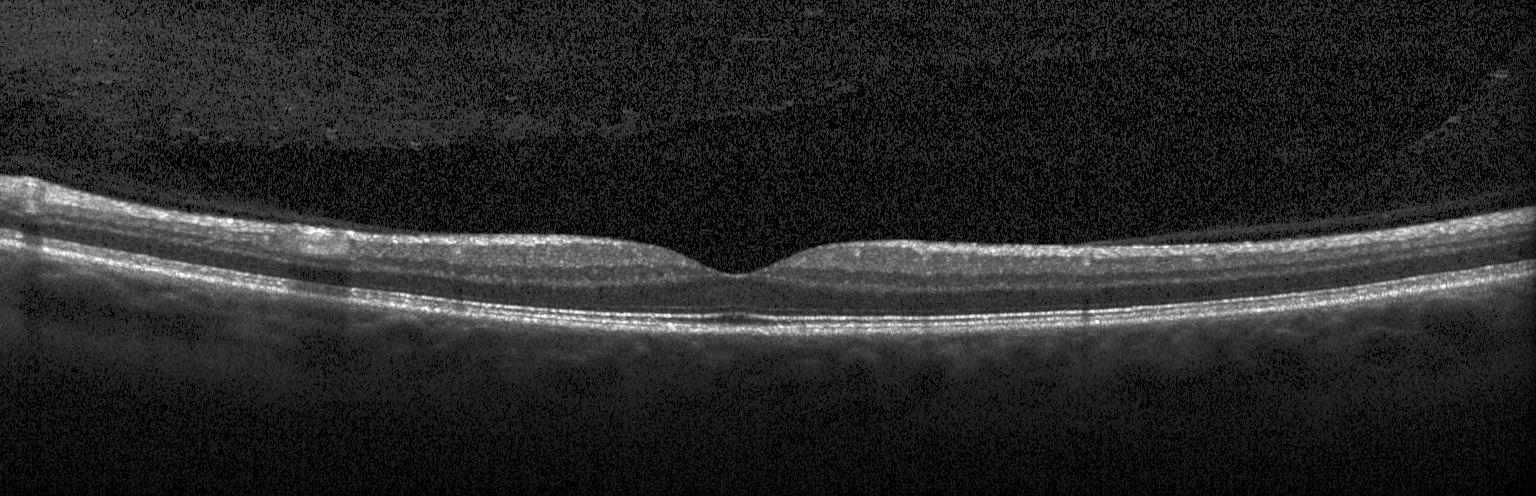 Optical coherence tomography B-scan · SD-OCT · instrument: Heidelberg Spectralis · horizontal scan through the fovea
Assessment: no CNV, no DME, and no drusen.